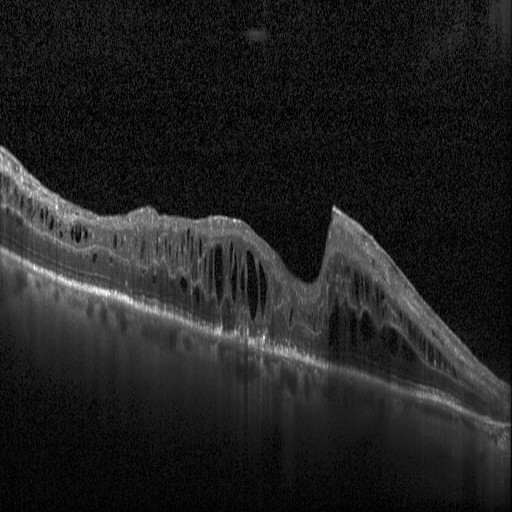 Optical coherence tomography B-scan, instrument: Heidelberg Spectralis. Finding: diabetic macular edema (DME).